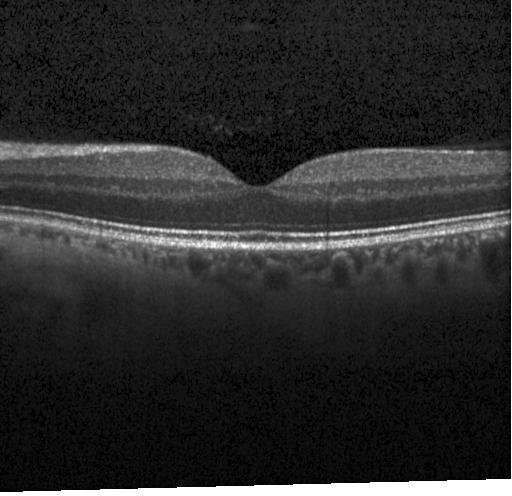

Diagnosis: no choroidal neovascularization, no diabetic macular edema, and no drusen.